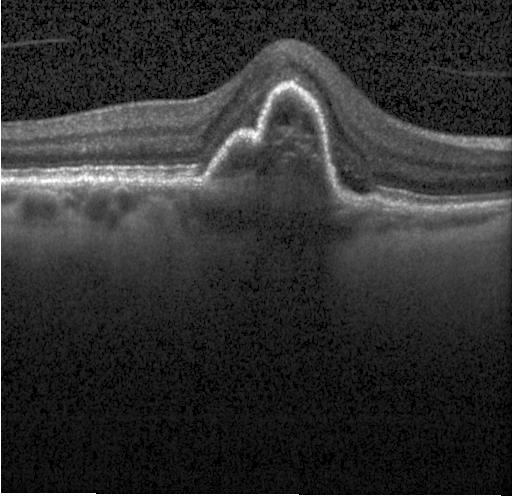 Optical coherence tomography scan
This B-scan demonstrates choroidal neovascularization.